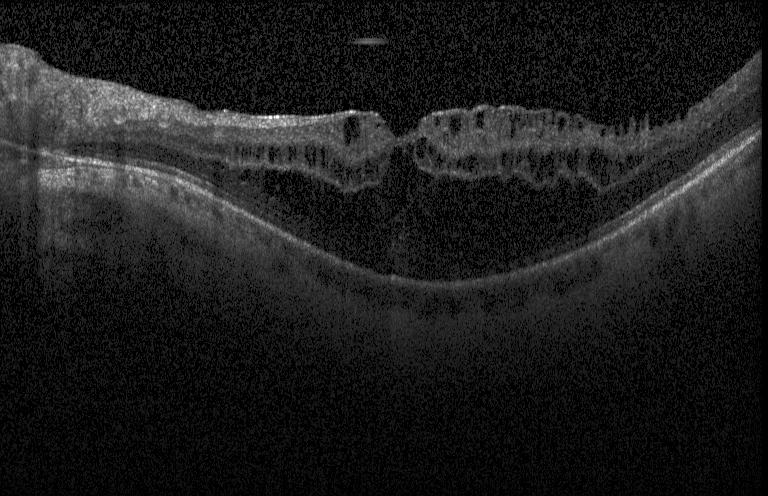

Retinal OCT B-scan. Instrument: Heidelberg Spectralis. The scan shows diabetic macular edema (DME).